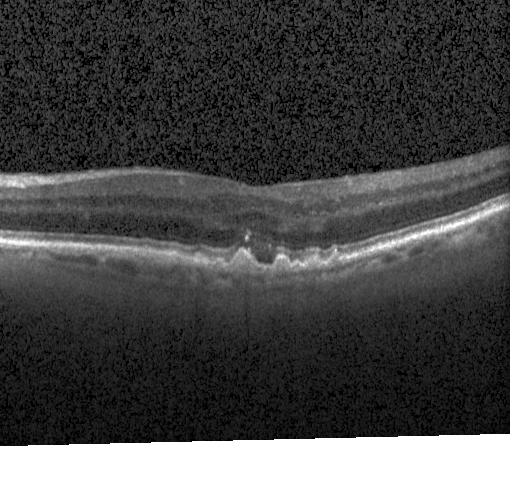
OCT finding: CNV.